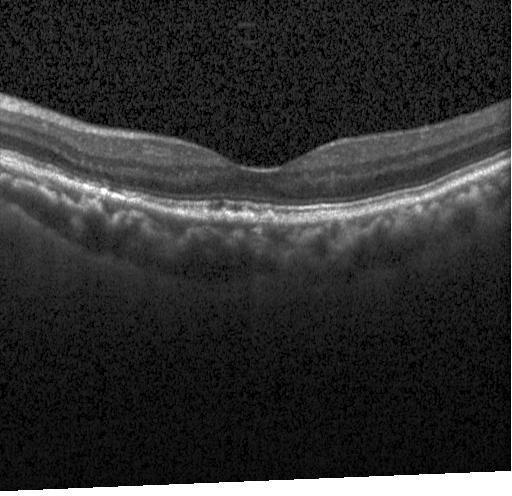

Retinal OCT B-scan. Spectral-domain OCT. Centered on the fovea. OCT finding: no evidence of CNV, DME, or drusen.